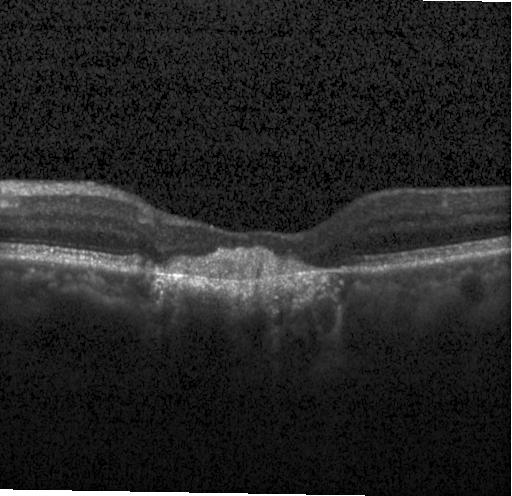 OCT finding: CNV.